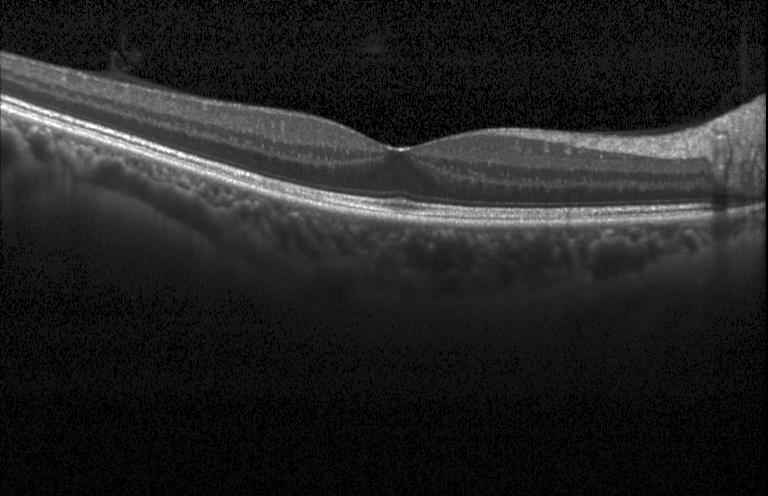 OCT B-scan, spectral-domain optical coherence tomography. Assessment: neither choroidal neovascularization, diabetic macular edema, nor drusen.